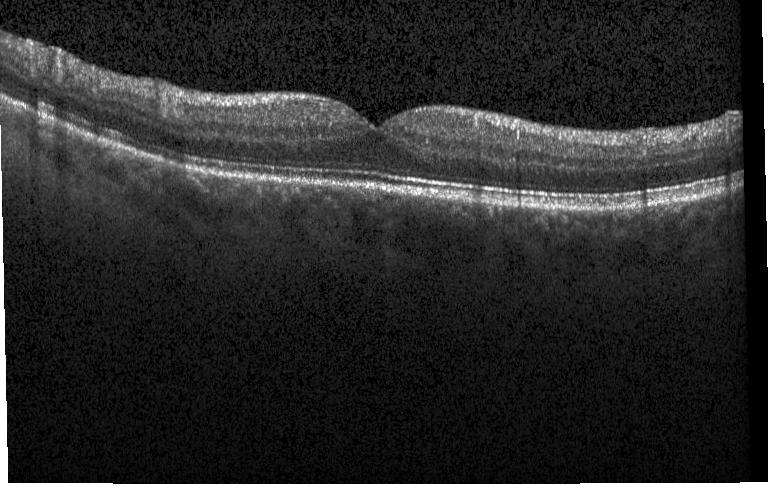

Optical coherence tomography scan
Assessment: no CNV, no DME, and no drusen.